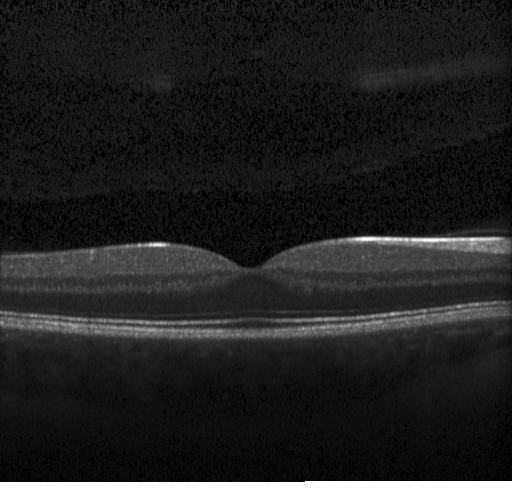

Centered on the fovea; acquired on a Heidelberg Spectralis; optical coherence tomography B-scan; SD-OCT — OCT finding: no CNV, no DME, and no drusen.